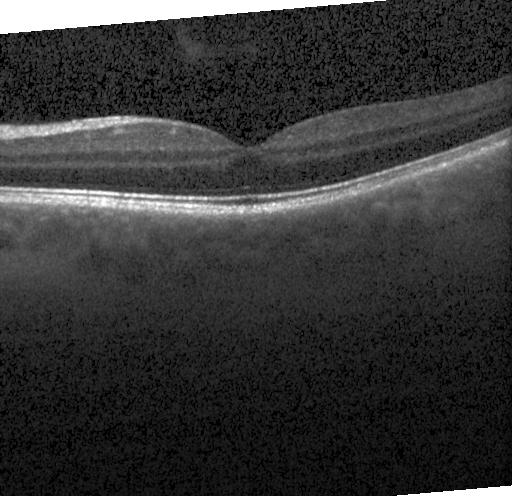

Centered on the fovea · SD-OCT · instrument: Heidelberg Spectralis · optical coherence tomography scan.
Macular OCT: no choroidal neovascularization, diabetic macular edema, or drusen.